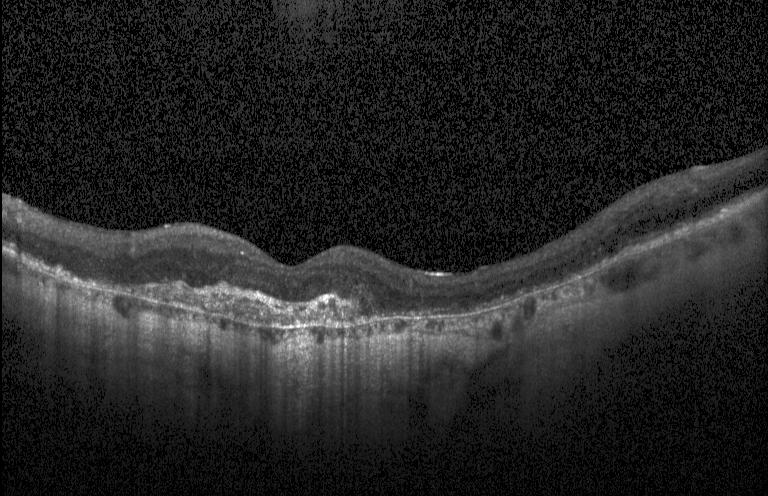 Centered on the fovea, spectral-domain OCT, optical coherence tomography B-scan. Finding: CNV.